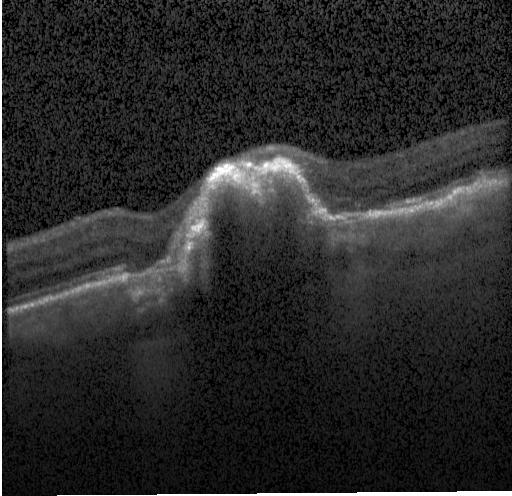

SD-OCT. Optical coherence tomography scan. Heidelberg Spectralis. A choroidal neovascular membrane.